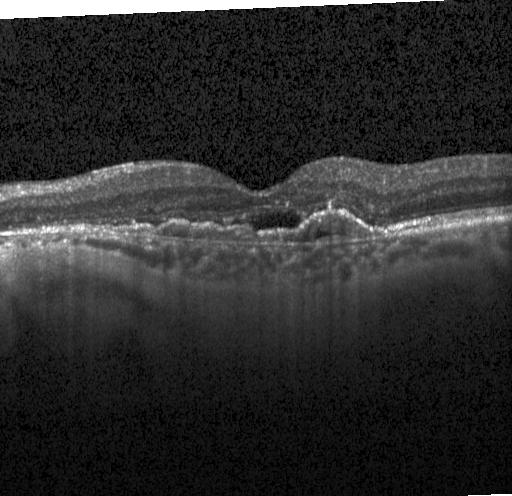
Heidelberg Spectralis OCT system, spectral-domain OCT, fovea-centered, optical coherence tomography B-scan — Diagnosis: a choroidal neovascular membrane.